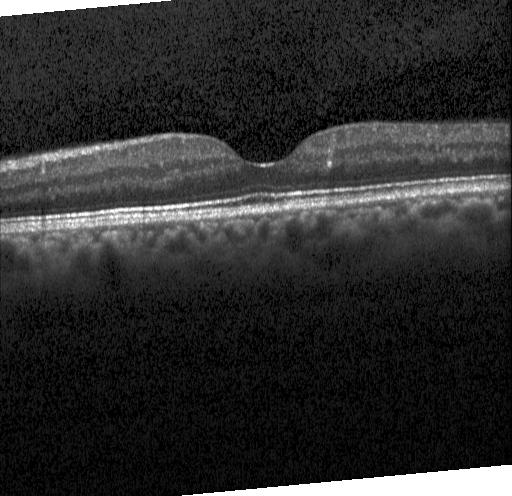
Retinal OCT cross-section, SD-OCT — Impression: neither choroidal neovascularization, diabetic macular edema, nor drusen.